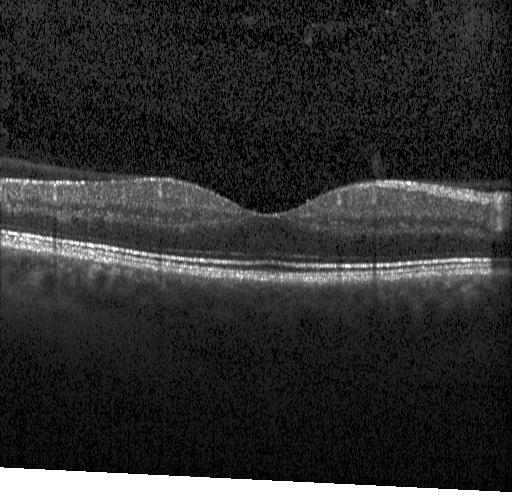

OCT B-scan. Macular OCT: no evidence of choroidal neovascularization, diabetic macular edema, or drusen.